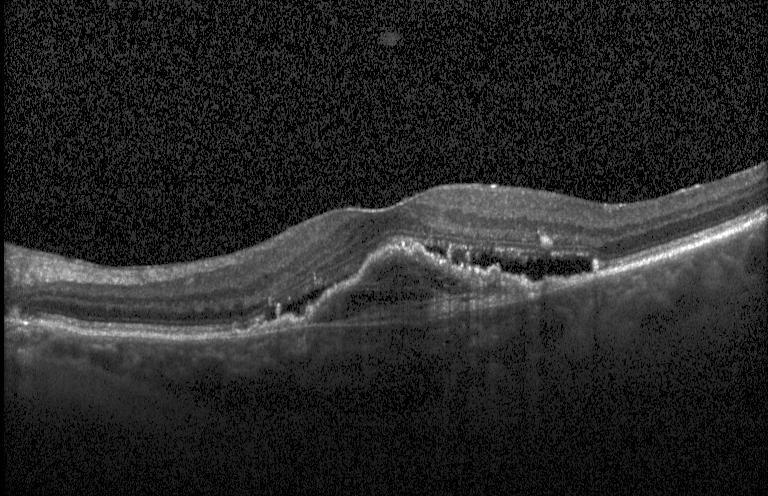 Spectral-domain OCT. OCT B-scan. Instrument: Heidelberg Spectralis. Macular scan. The scan shows choroidal neovascularization.